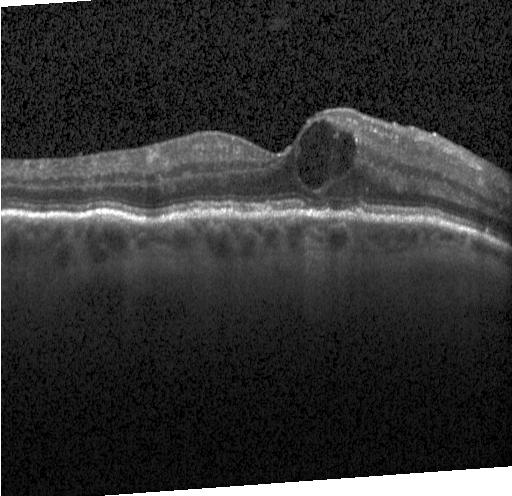

Optical coherence tomography B-scan; Heidelberg Spectralis OCT system; spectral-domain optical coherence tomography; macular scan — Macular OCT: a choroidal neovascular membrane.